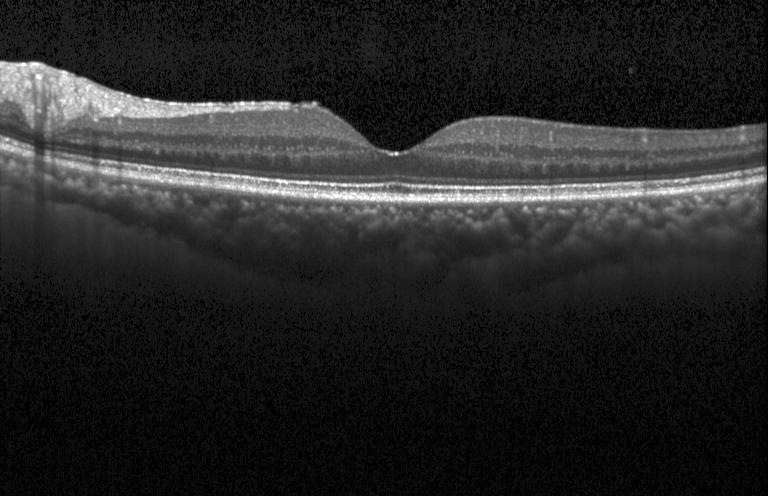

Spectral-domain OCT B-scan: no evidence of choroidal neovascularization, diabetic macular edema, or drusen.